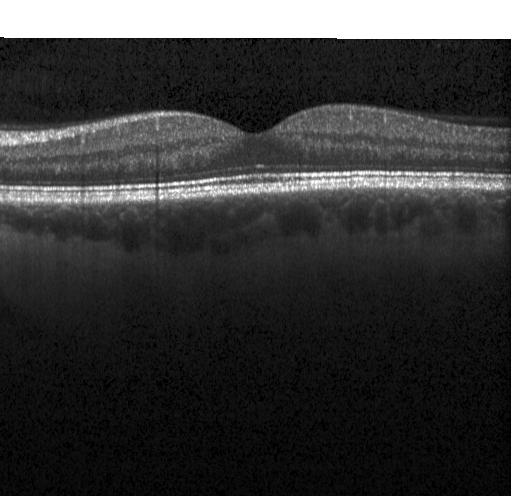 Diagnosis: no choroidal neovascularization, no diabetic macular edema, and no drusen.